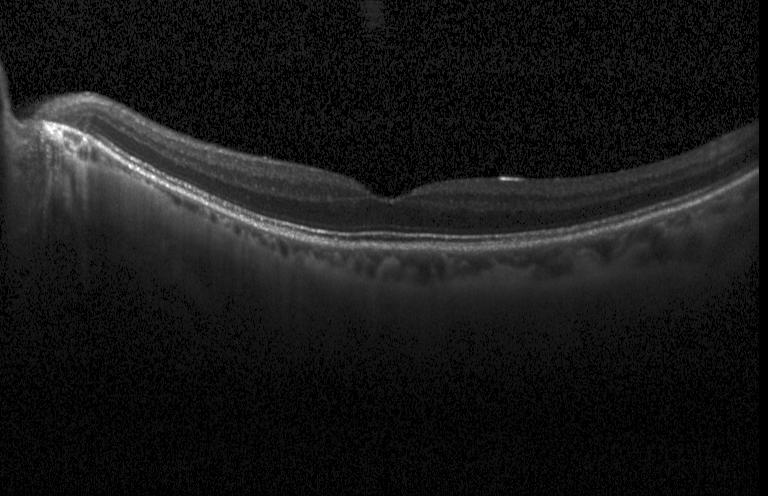

Impression: no choroidal neovascularization, no diabetic macular edema, and no drusen.